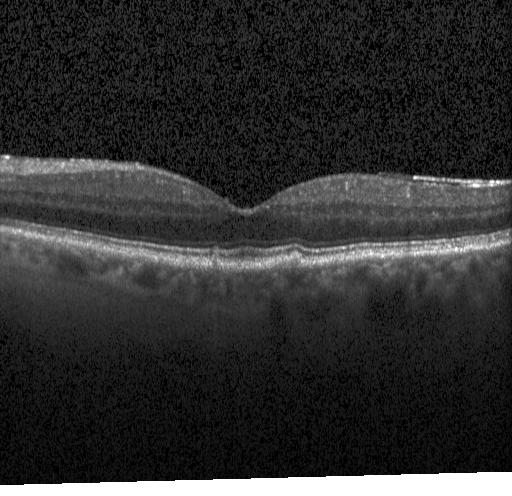

OCT B-scan showing sub-RPE drusenoid deposits.